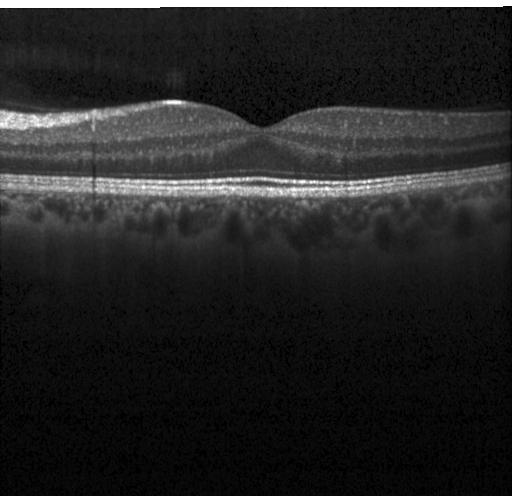 This B-scan demonstrates no evidence of choroidal neovascularization, diabetic macular edema, or drusen.